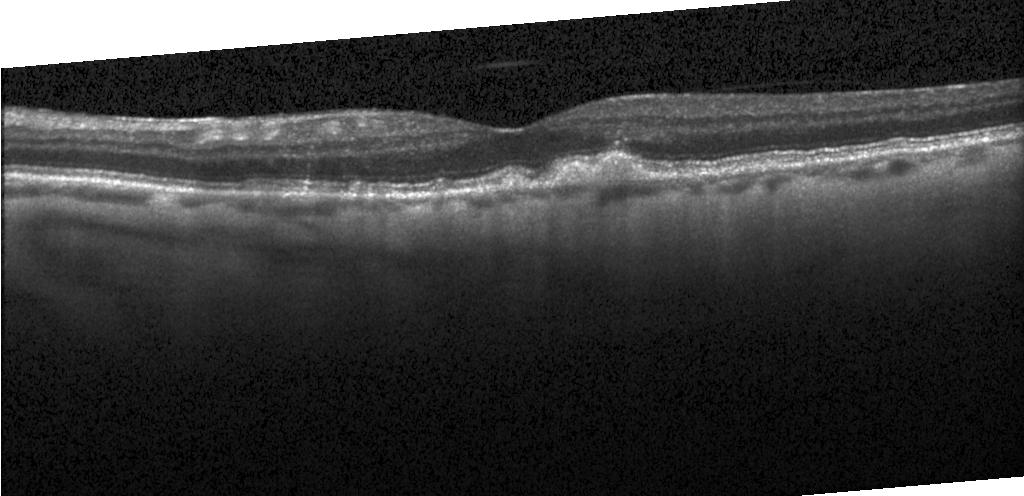 Impression: drusen.